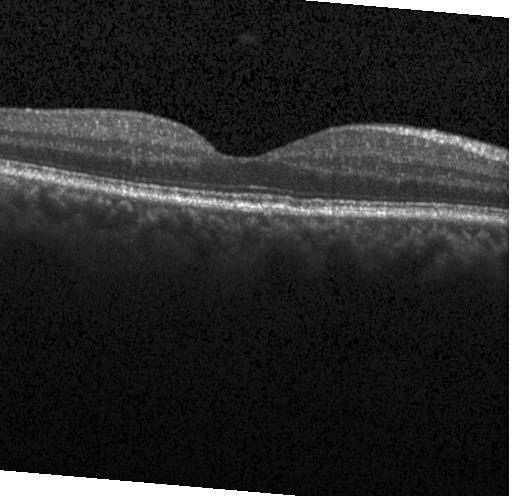 Retinal OCT cross-section. Macular scan
This B-scan demonstrates no choroidal neovascularization, diabetic macular edema, or drusen.